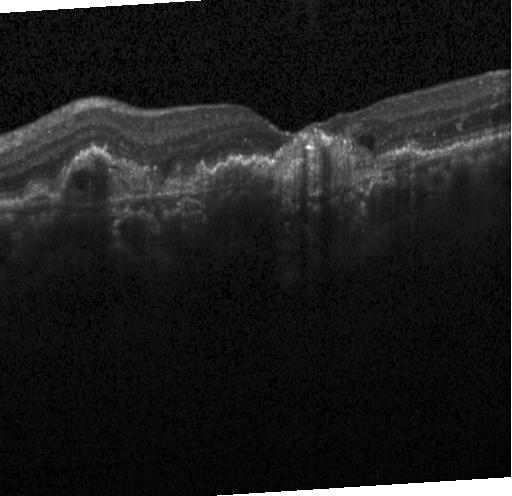

Spectral-domain optical coherence tomography; macular scan; retinal OCT cross-section — Macular OCT: choroidal neovascularization (CNV).